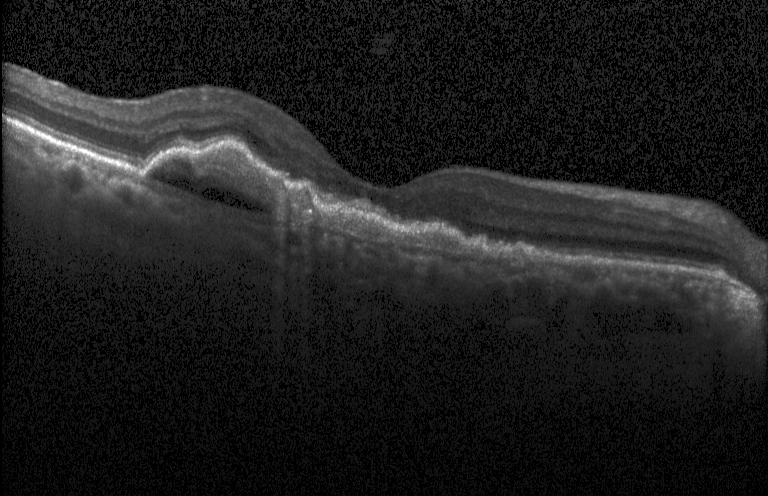

Retinal OCT B-scan, horizontal scan through the fovea, acquired on a Heidelberg Spectralis
Dx: choroidal neovascularization (CNV).